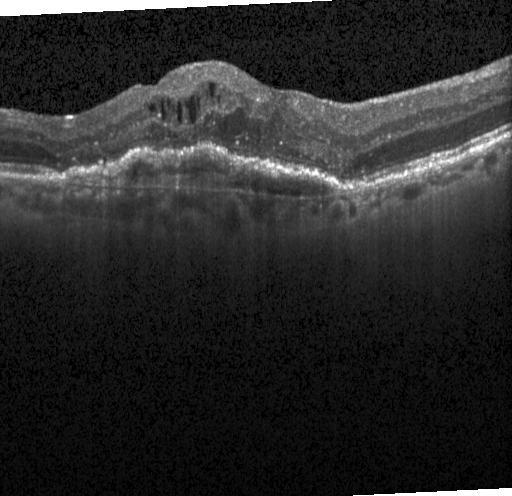 SD-OCT; centered on the fovea; acquired on a Heidelberg Spectralis; retinal OCT cross-section — Macular OCT: a choroidal neovascular membrane.